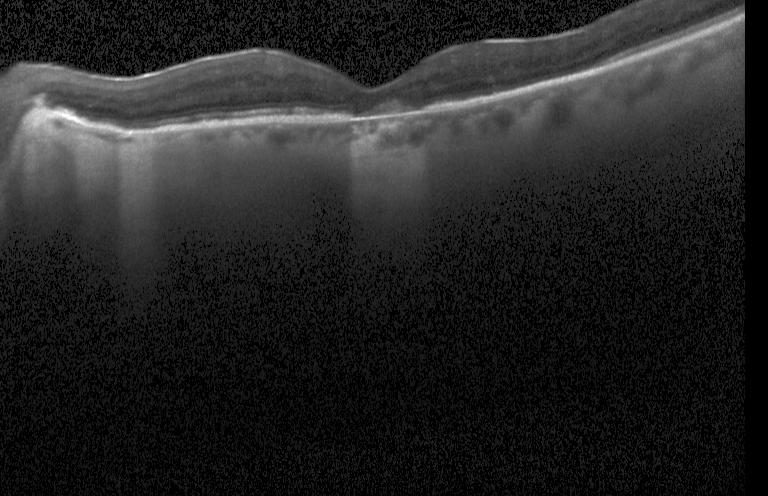
Heidelberg Spectralis, OCT B-scan. Assessment: a choroidal neovascular membrane.